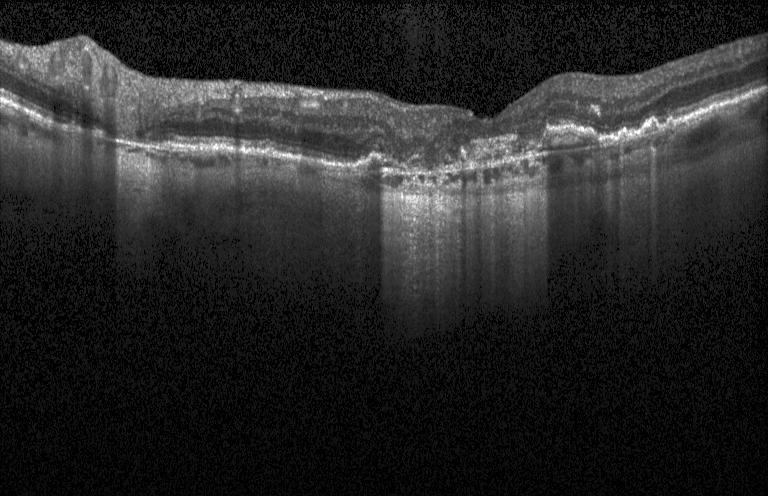

Heidelberg Spectralis OCT system. Retinal OCT cross-section. Spectral-domain OCT. The scan shows choroidal neovascularization.